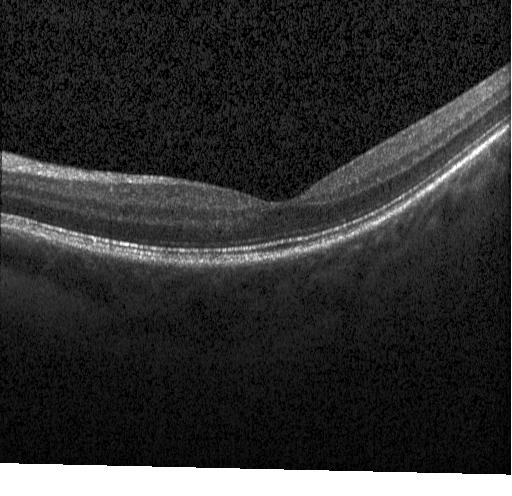
Heidelberg Spectralis OCT system, OCT line scan, centered on the fovea.
Impression: no choroidal neovascularization, diabetic macular edema, or drusen.